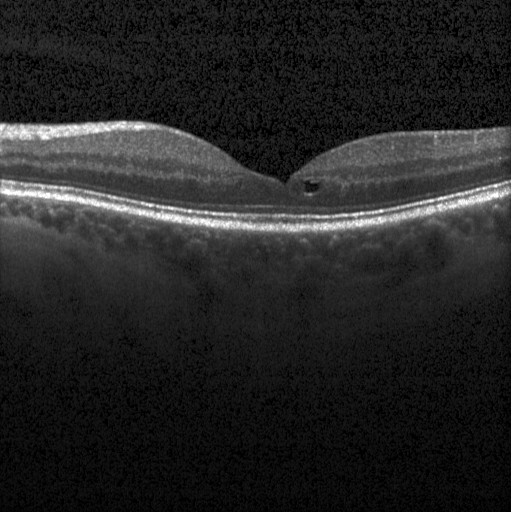
The scan shows diabetic macular edema (DME).